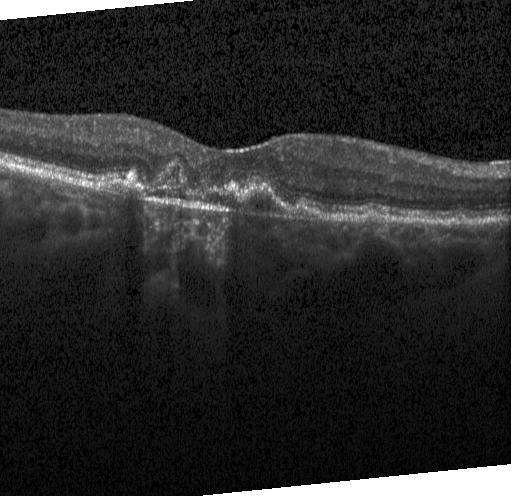

Impression: choroidal neovascularization (CNV).